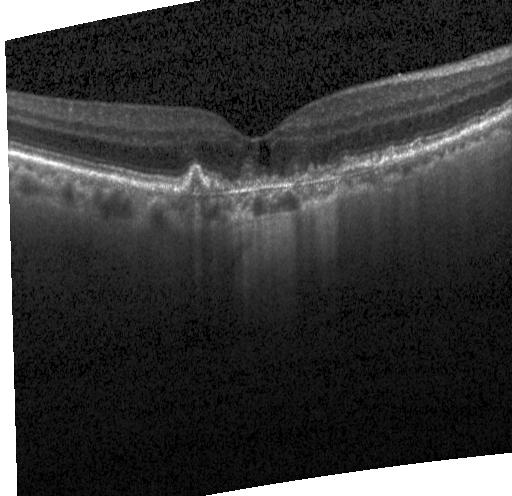
Retinal OCT cross-section showing a choroidal neovascular membrane.